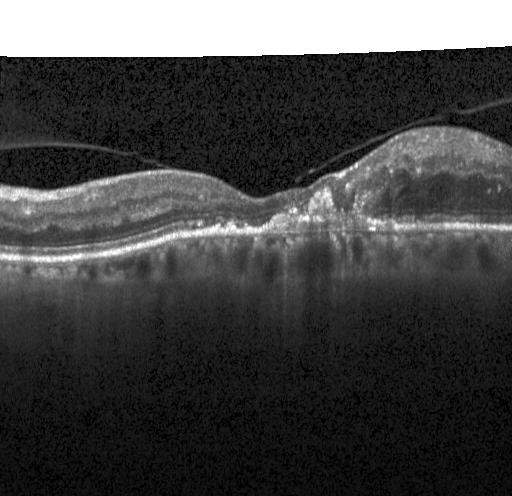 Centered on the fovea · retinal OCT cross-section · Heidelberg Spectralis. Impression: CNV.